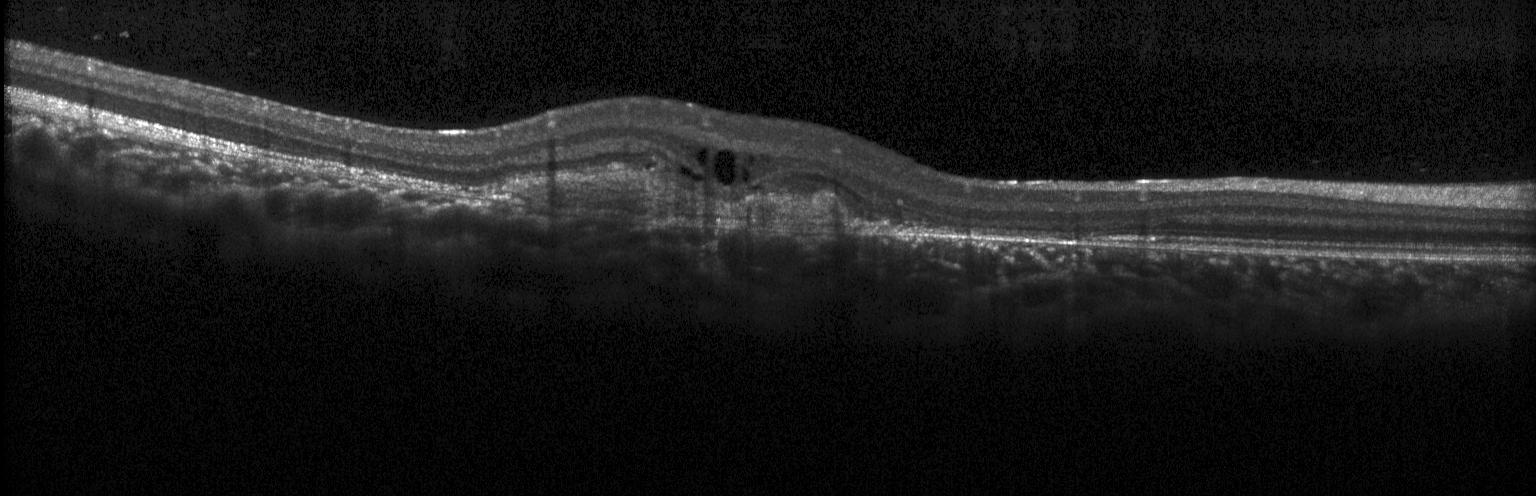

OCT line scan; macular scan; Heidelberg Spectralis — This B-scan demonstrates CNV.